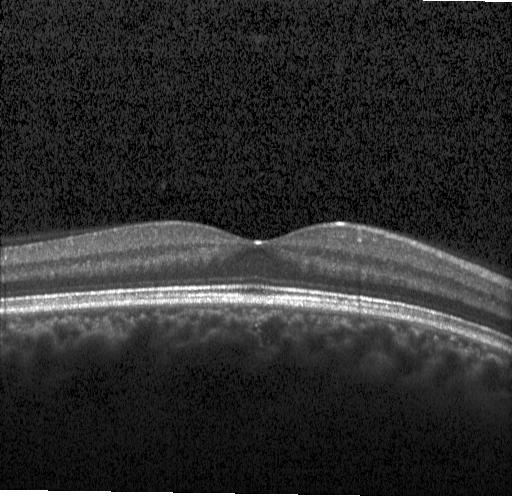 Macular OCT: no choroidal neovascularization, no diabetic macular edema, and no drusen.